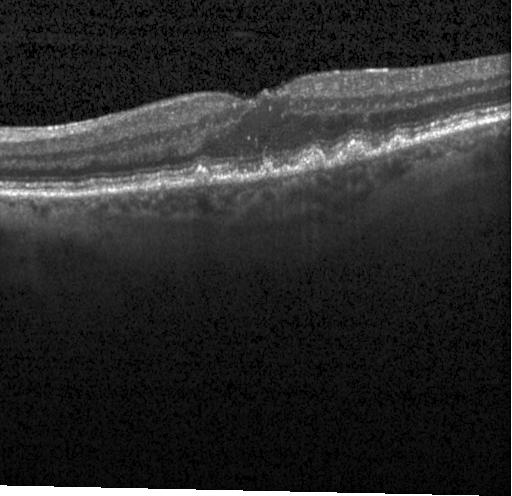
Optical coherence tomography B-scan; horizontal scan through the fovea; acquired on a Heidelberg Spectralis — Diagnosis: drusen.